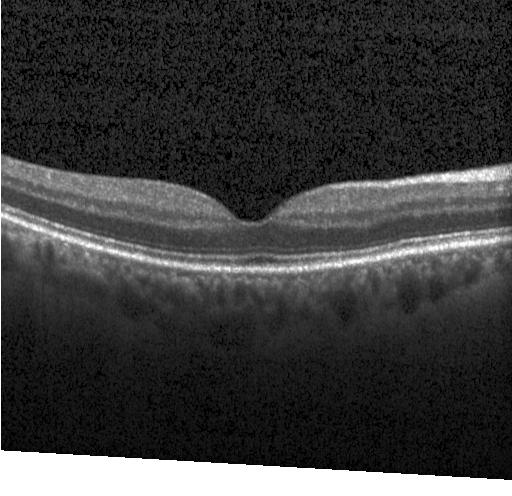
Optical coherence tomography B-scan — Finding: no evidence of choroidal neovascularization, diabetic macular edema, or drusen.